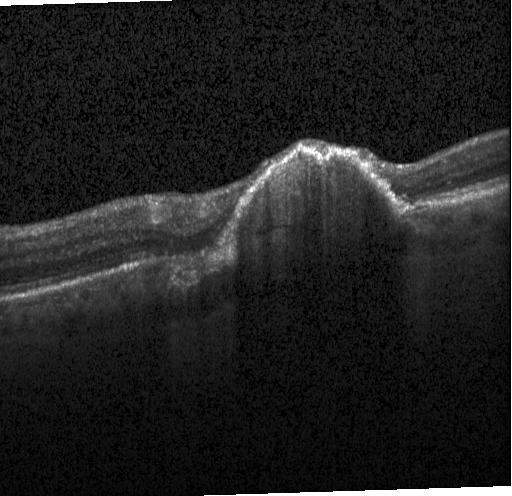
Diagnosis: a choroidal neovascular membrane.